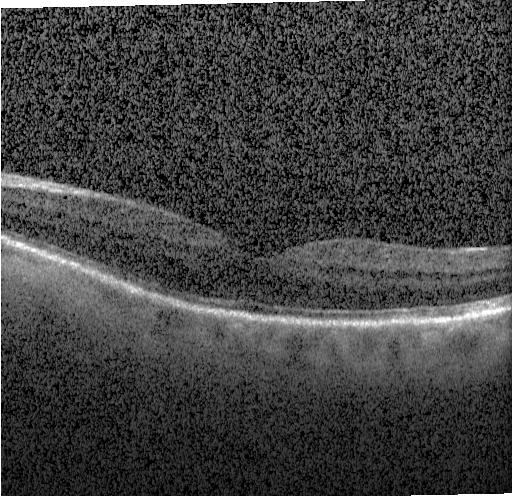

Horizontal scan through the fovea. Heidelberg Spectralis OCT system. Optical coherence tomography scan. SD-OCT.
This B-scan demonstrates no evidence of choroidal neovascularization, diabetic macular edema, or drusen.